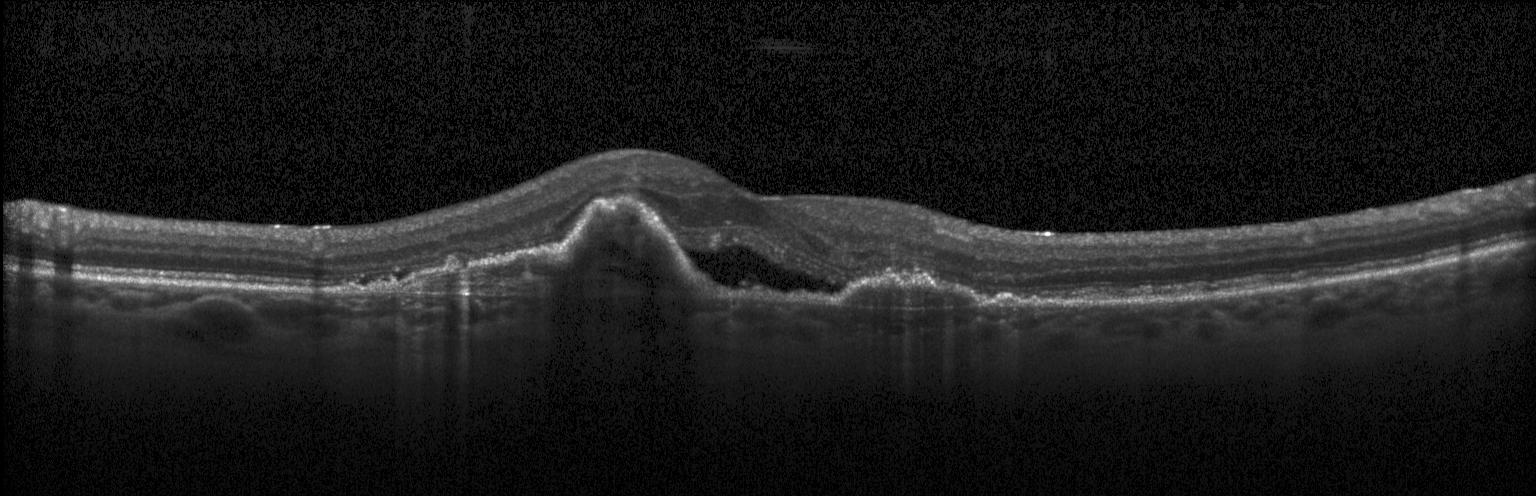

Finding: choroidal neovascularization.